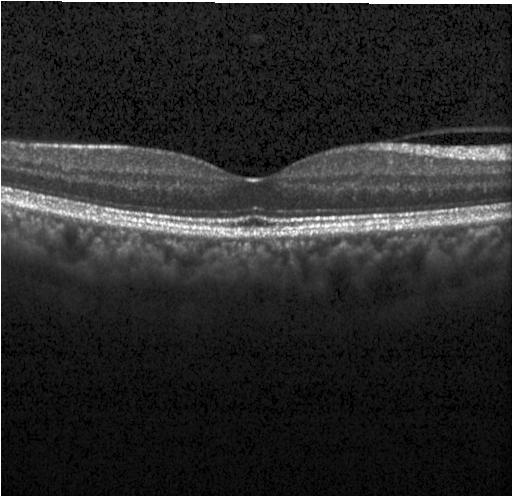

OCT finding: no evidence of choroidal neovascularization, diabetic macular edema, or drusen.